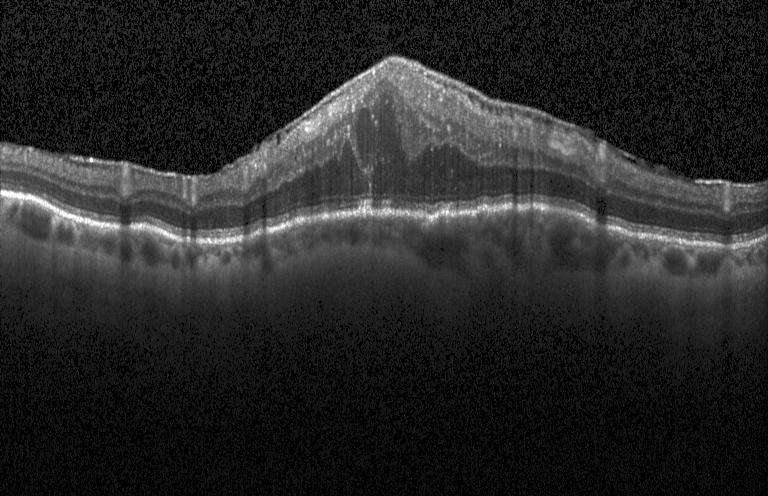

OCT scan showing DME.